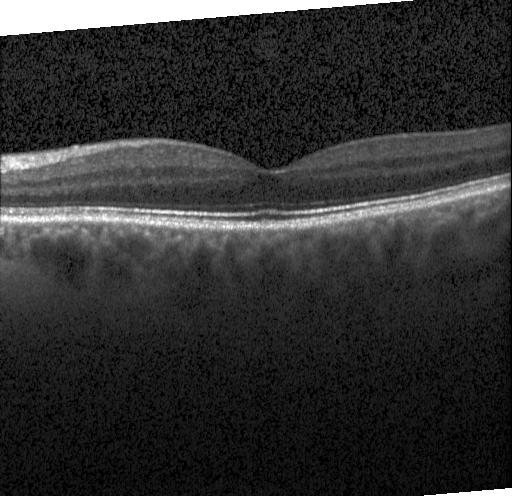

OCT B-scan showing neither choroidal neovascularization, diabetic macular edema, nor drusen.